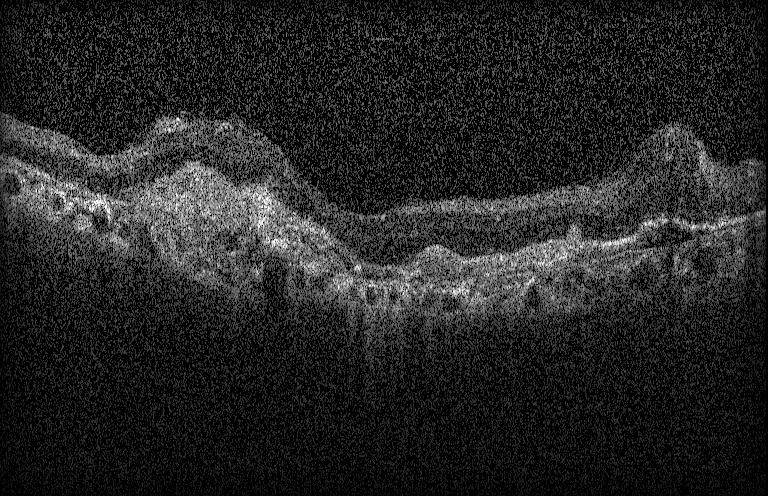 OCT B-scan showing CNV.